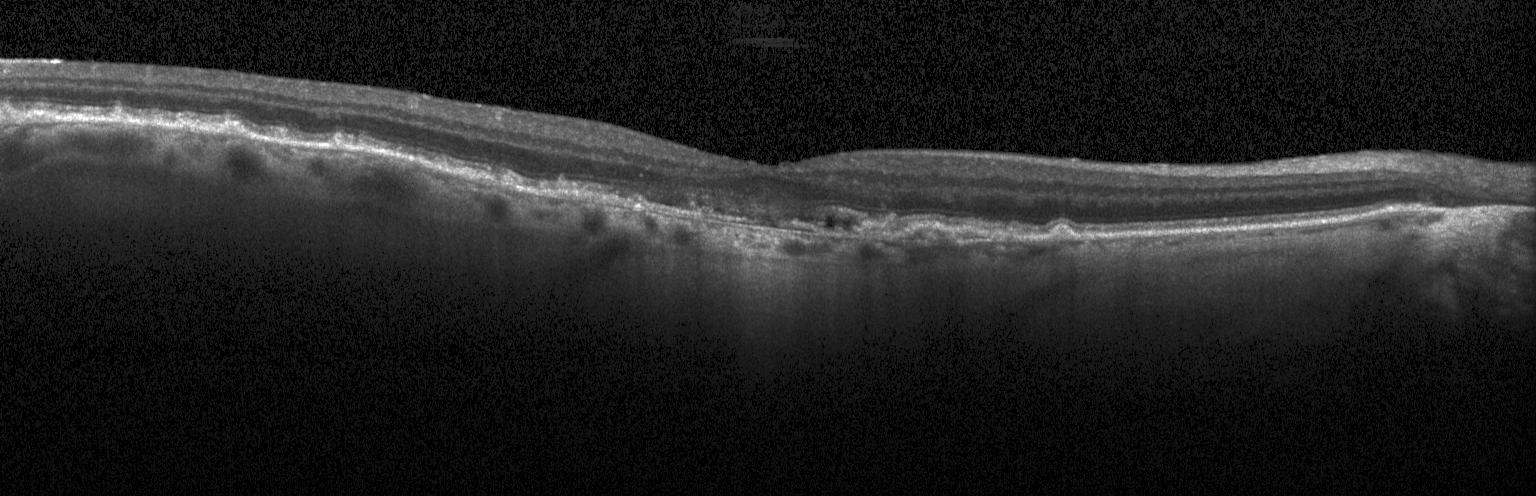 OCT scan showing CNV.